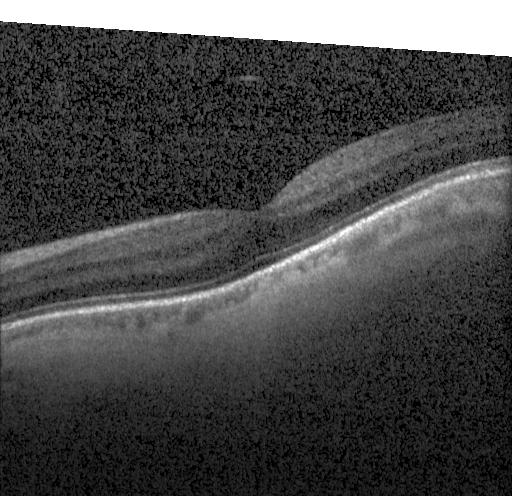
OCT B-scan — Diagnosis: no evidence of choroidal neovascularization, diabetic macular edema, or drusen.